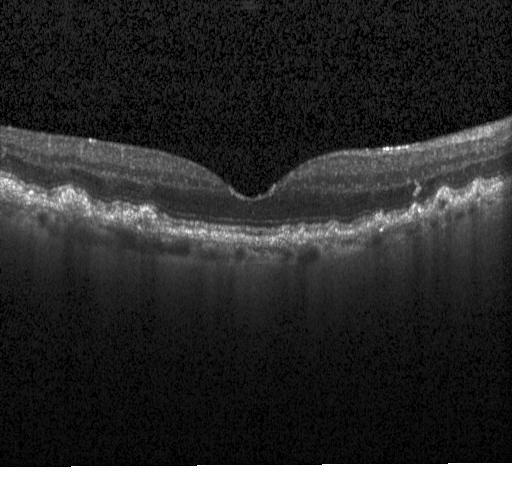 Spectral-domain OCT; OCT B-scan; acquired on a Heidelberg Spectralis — Dx: drusen.